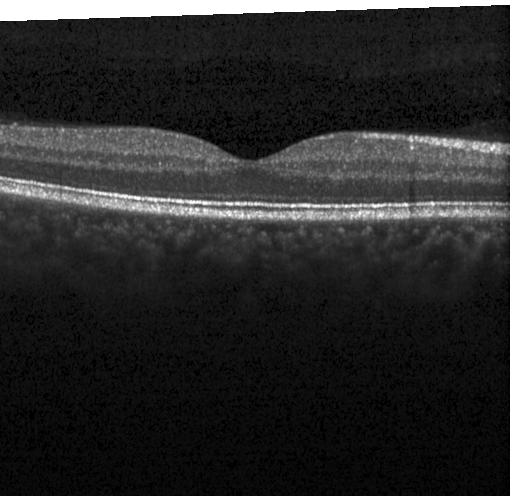 Horizontal scan through the fovea. Heidelberg Spectralis. Optical coherence tomography B-scan — Assessment: no choroidal neovascularization, no diabetic macular edema, and no drusen.